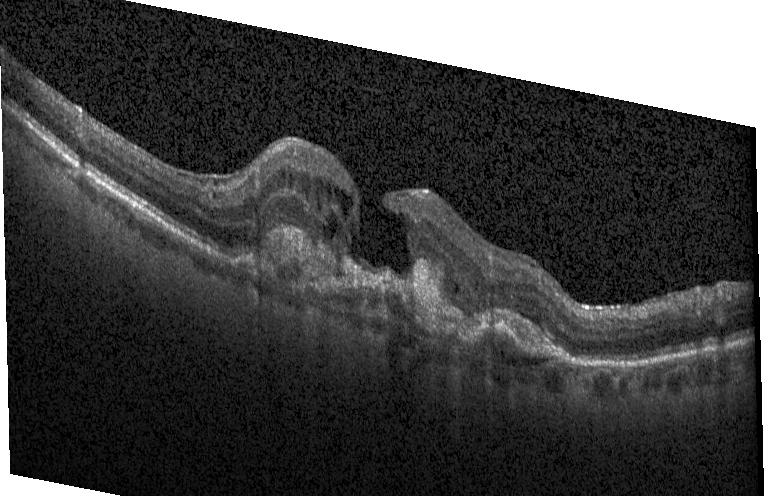

Dx: a choroidal neovascular membrane.